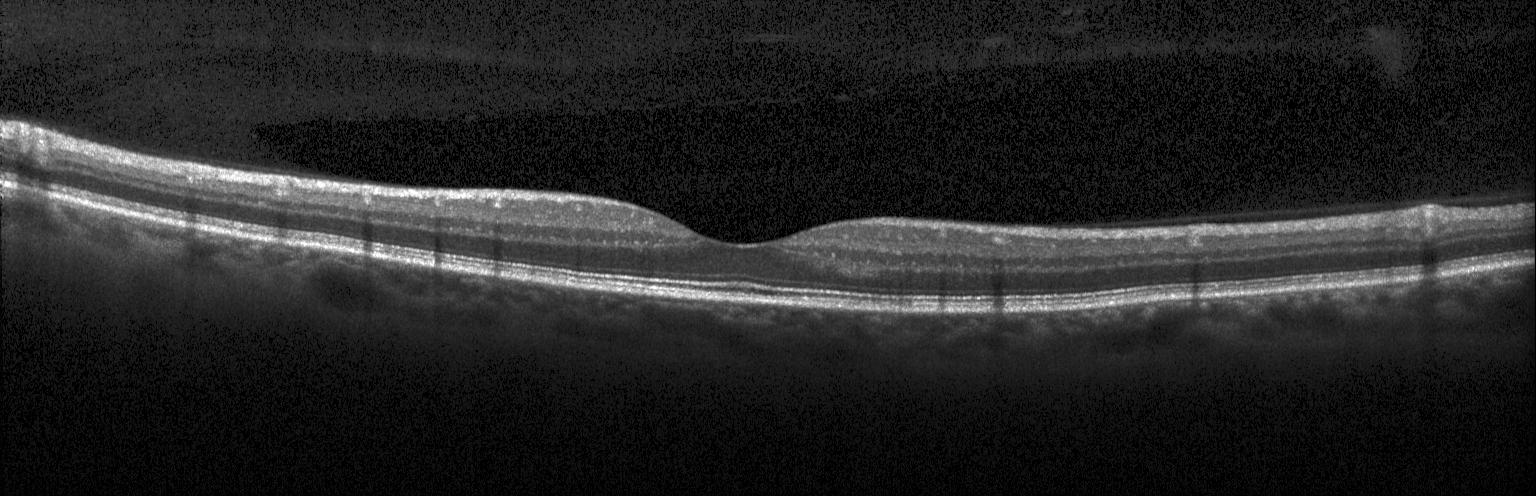

No evidence of CNV, DME, or drusen.